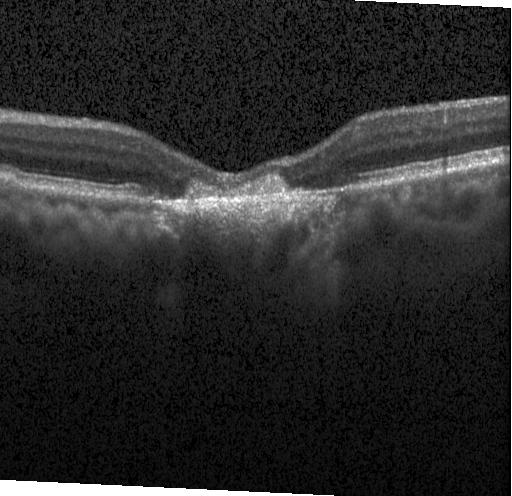 OCT line scan. Dx: a choroidal neovascular membrane.